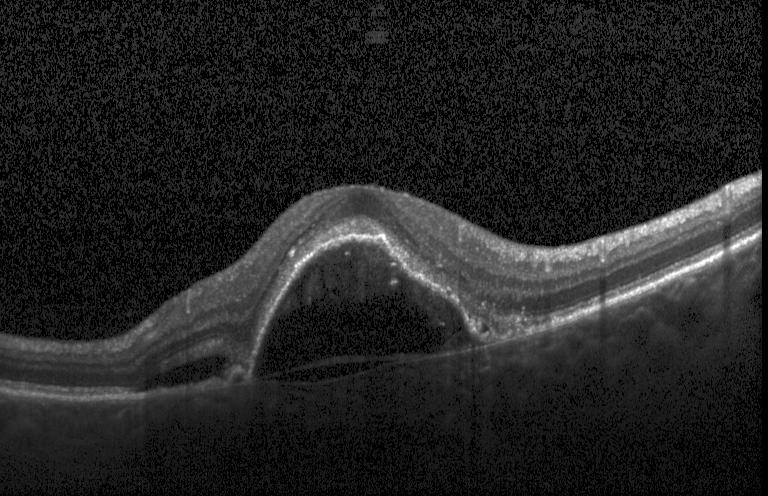 Dx: CNV.